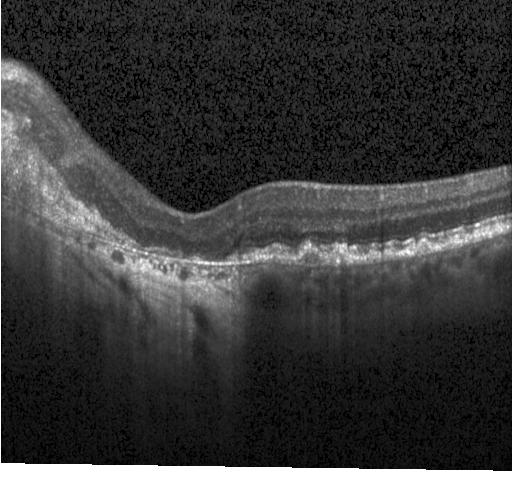
Assessment: CNV.